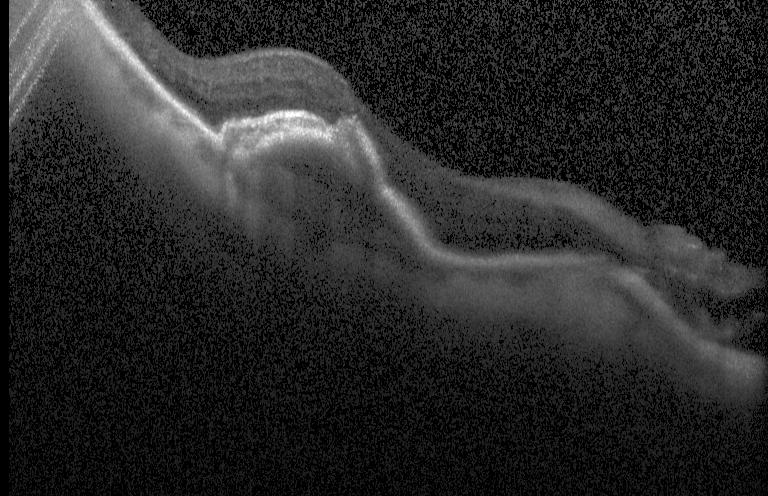

Impression: a choroidal neovascular membrane.